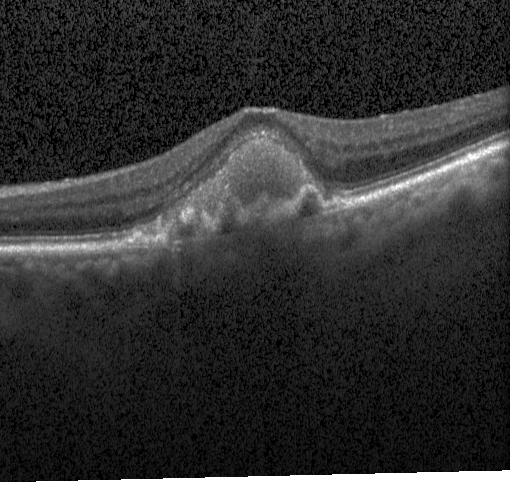

OCT B-scan, centered on the fovea, Heidelberg Spectralis OCT system, spectral-domain optical coherence tomography.
This B-scan demonstrates a choroidal neovascular membrane.